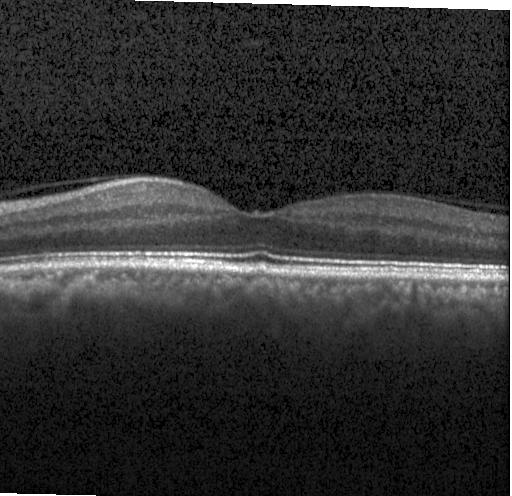
Spectral-domain optical coherence tomography; OCT B-scan; Heidelberg Spectralis. Diagnosis: no choroidal neovascularization, diabetic macular edema, or drusen.